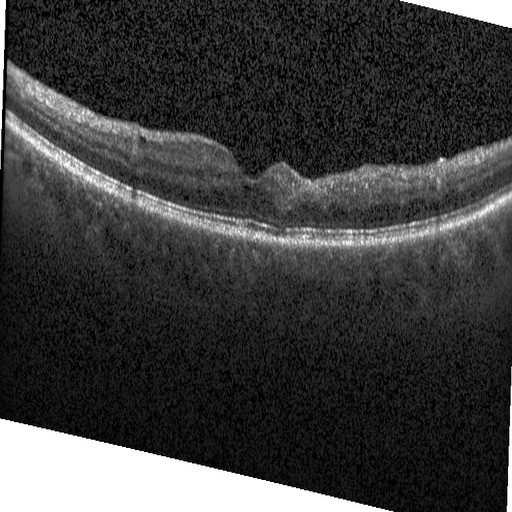
Retinal OCT B-scan.
Diagnosis: diabetic macular edema (DME).